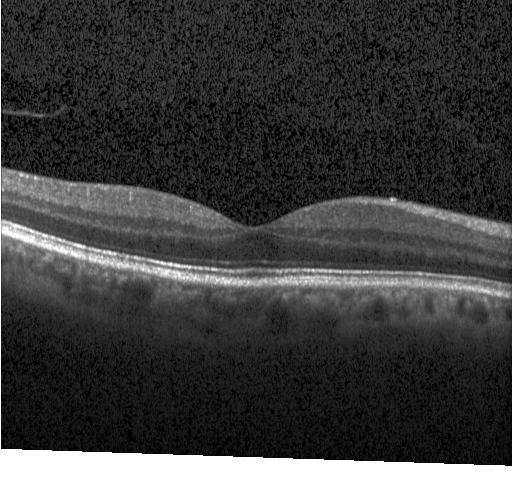

Retinal OCT cross-section. OCT finding: no choroidal neovascularization, diabetic macular edema, or drusen.